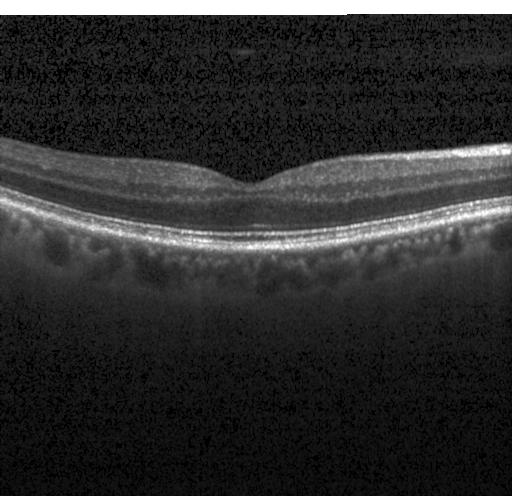
Retinal OCT cross-section — This B-scan demonstrates no choroidal neovascularization, diabetic macular edema, or drusen.